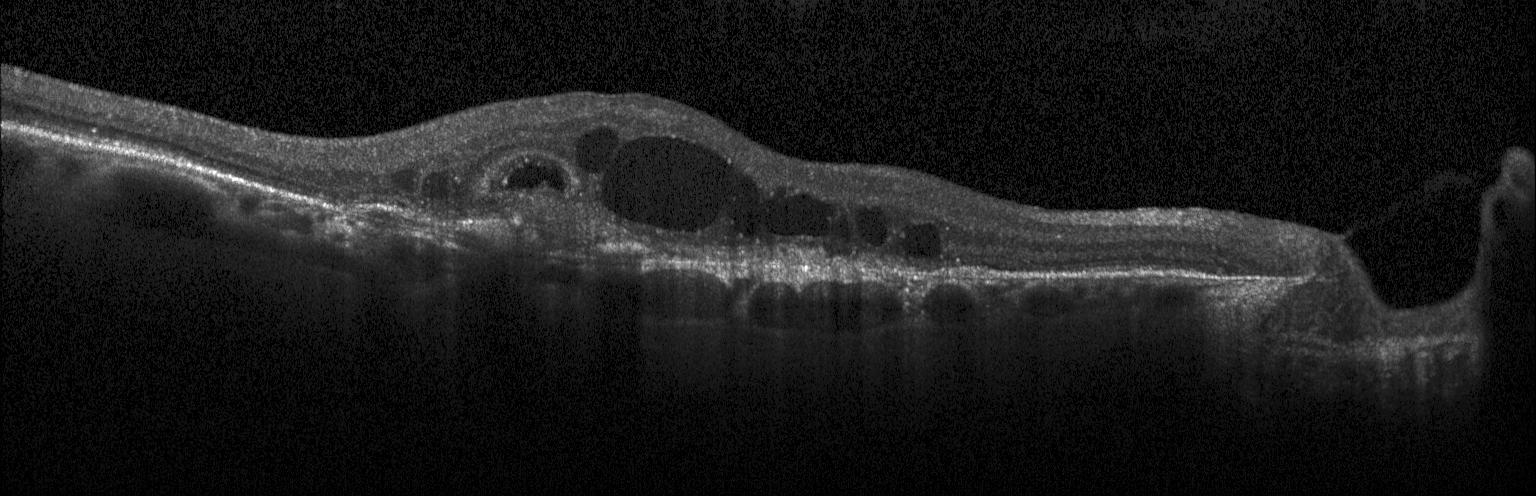

OCT B-scan showing choroidal neovascularization.